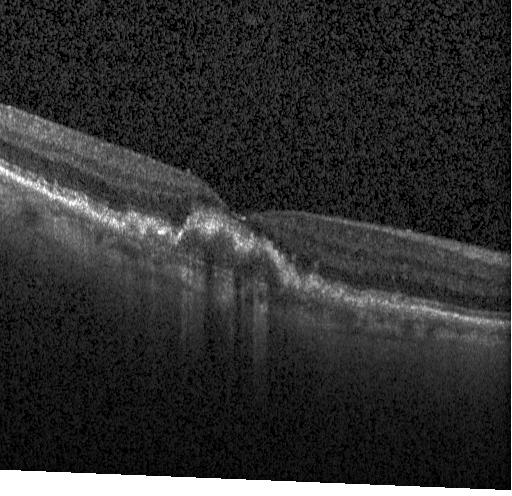
Heidelberg Spectralis OCT system. Horizontal scan through the fovea. Retinal OCT cross-section. Spectral-domain OCT — Diagnosis: a choroidal neovascular membrane.